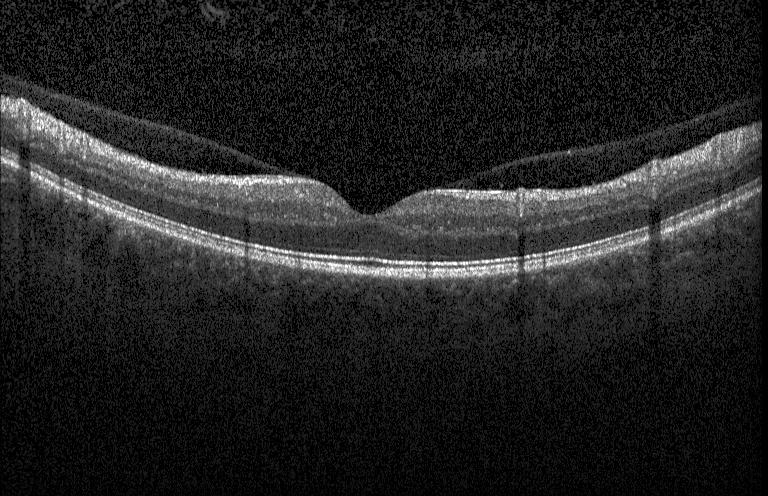 OCT B-scan showing no CNV, no DME, and no drusen.